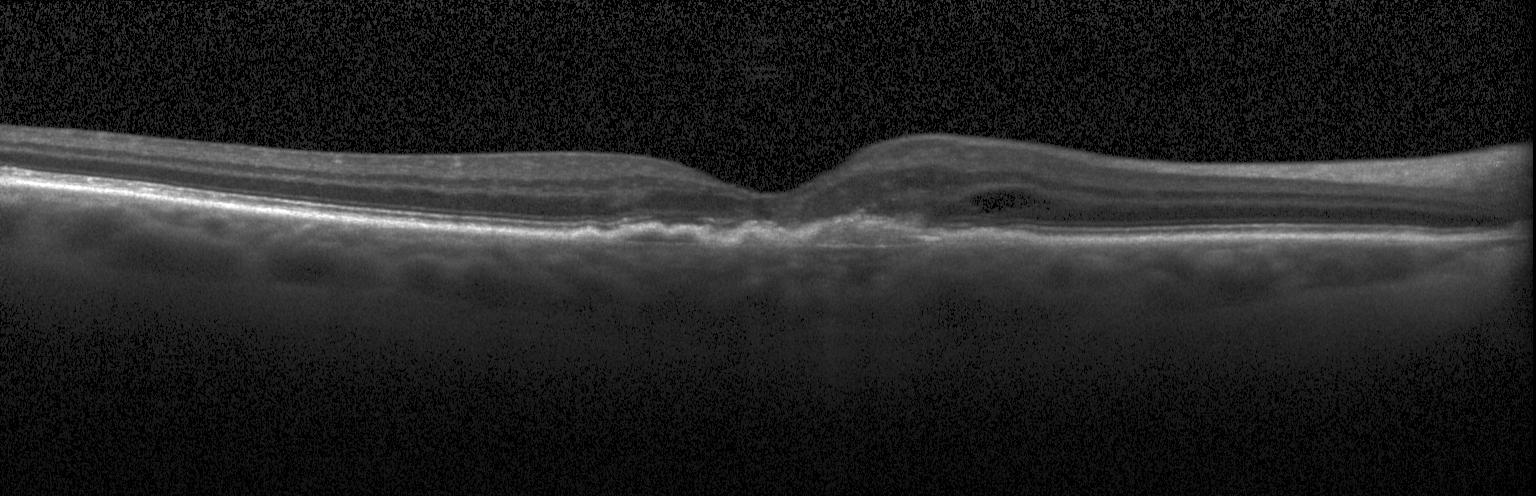
Instrument: Heidelberg Spectralis; optical coherence tomography B-scan.
A choroidal neovascular membrane.